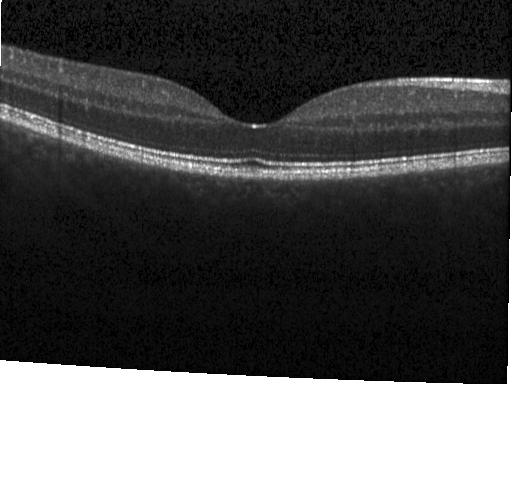 Optical coherence tomography scan. Instrument: Heidelberg Spectralis — Impression: no evidence of CNV, DME, or drusen.